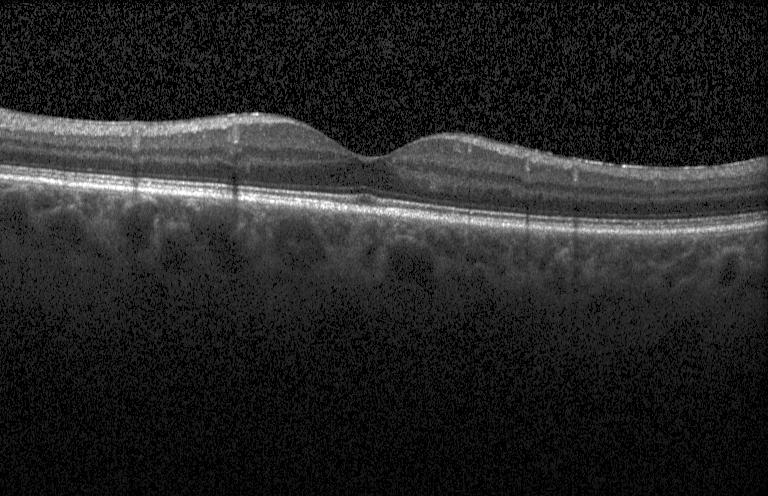
Centered on the fovea, spectral-domain OCT, Heidelberg Spectralis OCT system, retinal OCT B-scan. Finding: no evidence of CNV, DME, or drusen.